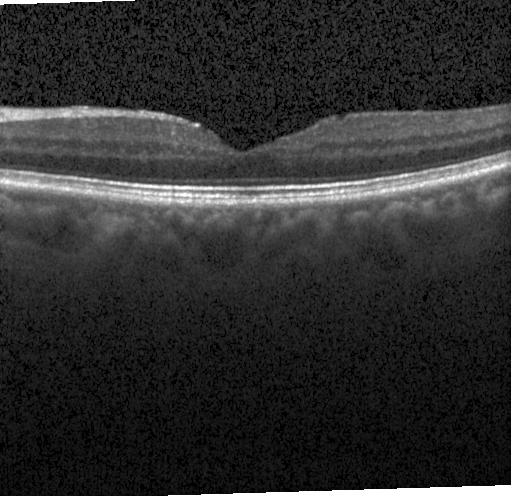

Fovea-centered · SD-OCT · optical coherence tomography B-scan · instrument: Heidelberg Spectralis
The scan shows no choroidal neovascularization, no diabetic macular edema, and no drusen.